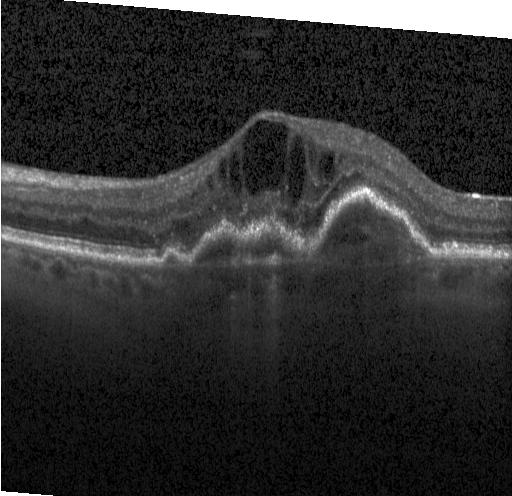
Optical coherence tomography B-scan — OCT finding: CNV.